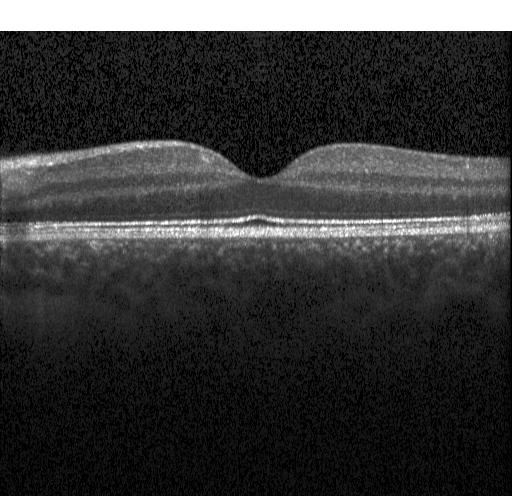 Acquired on a Heidelberg Spectralis · retinal OCT cross-section · centered on the fovea · SD-OCT
The scan shows neither choroidal neovascularization, diabetic macular edema, nor drusen.